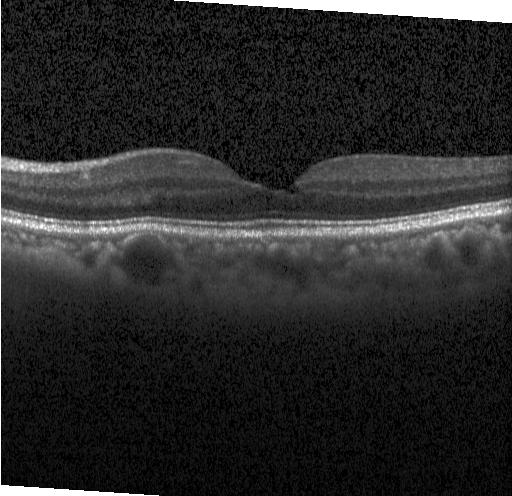
Fovea-centered, spectral-domain optical coherence tomography, instrument: Heidelberg Spectralis, OCT B-scan
Impression: neither CNV, DME, nor drusen.